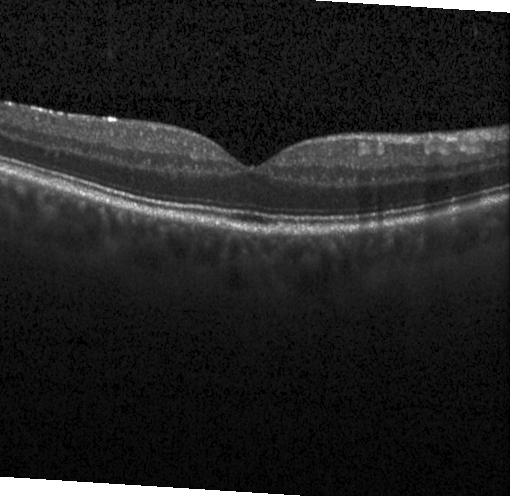
Horizontal scan through the fovea · spectral-domain optical coherence tomography · retinal OCT cross-section. Impression: no CNV, DME, or drusen.